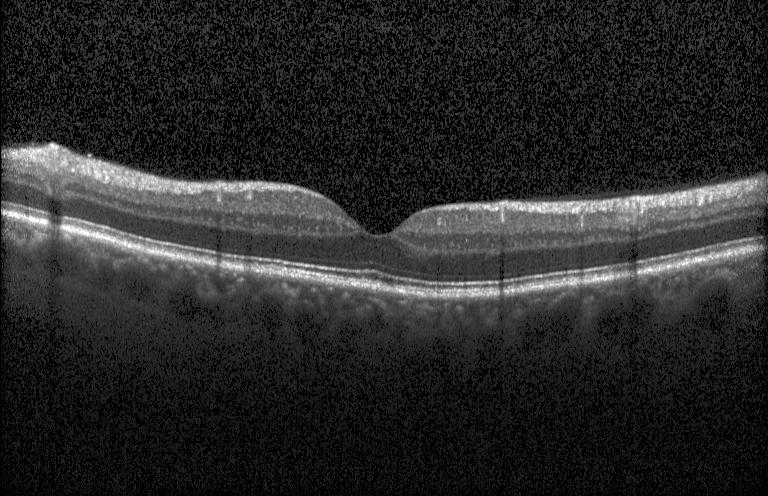 Horizontal scan through the fovea · optical coherence tomography scan · Heidelberg Spectralis OCT system · SD-OCT. Neither choroidal neovascularization, diabetic macular edema, nor drusen.